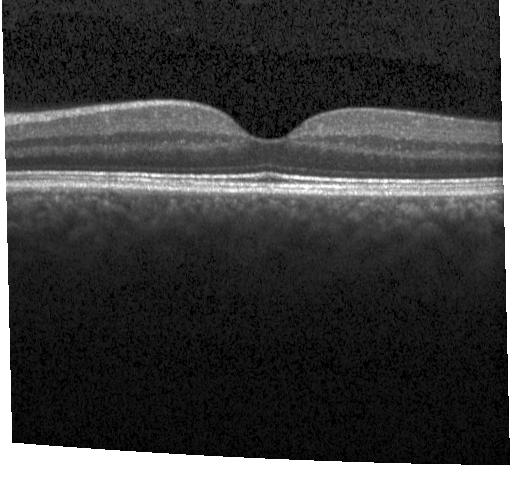

Horizontal scan through the fovea; Heidelberg Spectralis OCT system; retinal OCT cross-section; SD-OCT. No choroidal neovascularization, no diabetic macular edema, and no drusen.